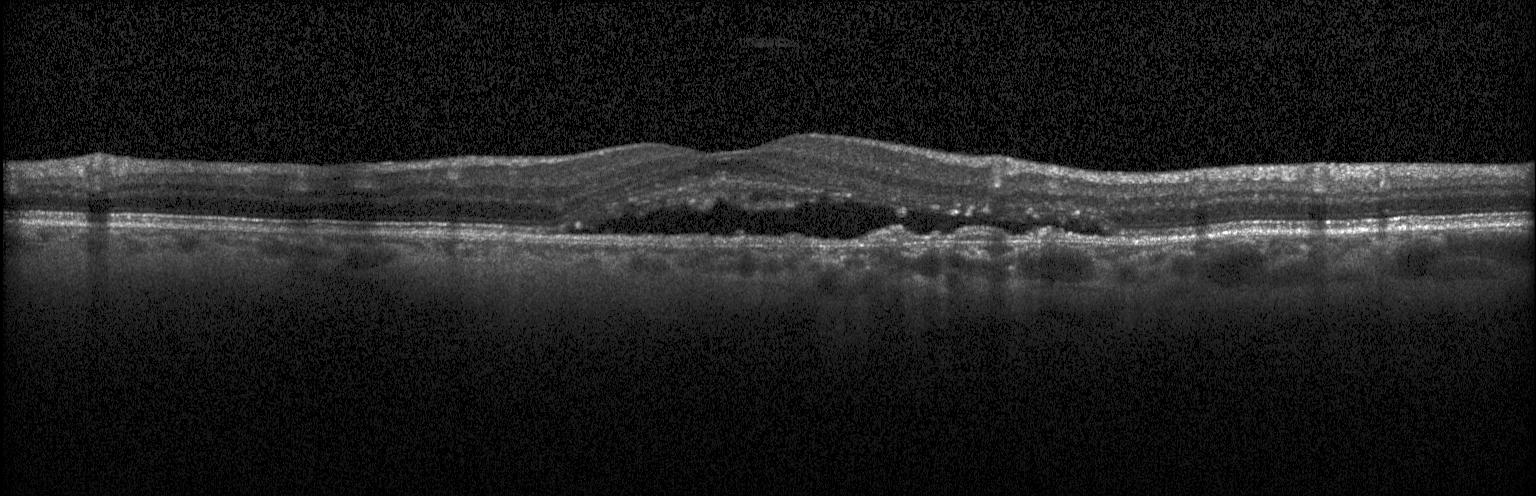
Horizontal scan through the fovea; spectral-domain optical coherence tomography; optical coherence tomography B-scan; instrument: Heidelberg Spectralis.
Finding: a choroidal neovascular membrane.